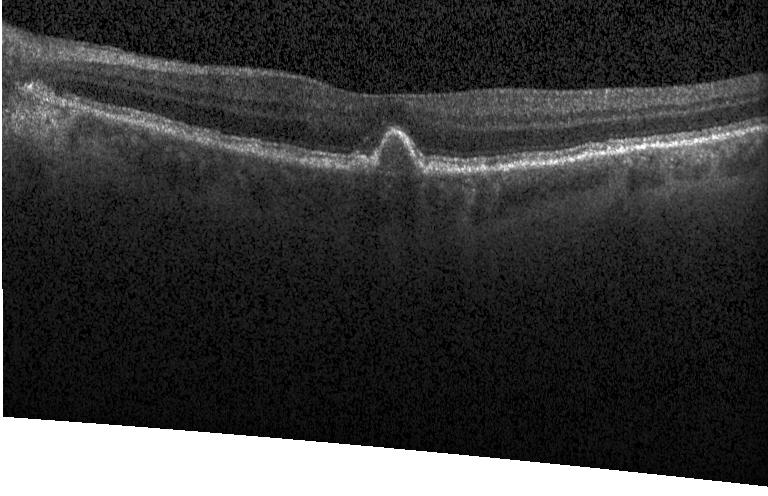

Retinal OCT B-scan
Assessment: drusen.